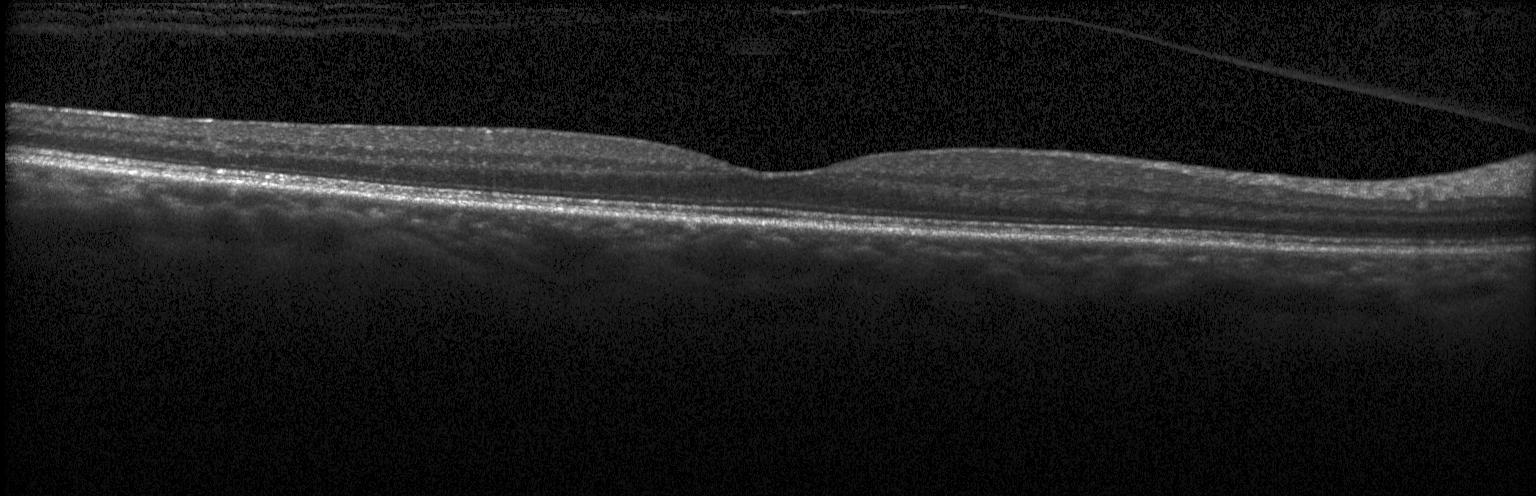

Centered on the fovea; optical coherence tomography scan; spectral-domain OCT; Heidelberg Spectralis.
Macular OCT: no choroidal neovascularization, diabetic macular edema, or drusen.